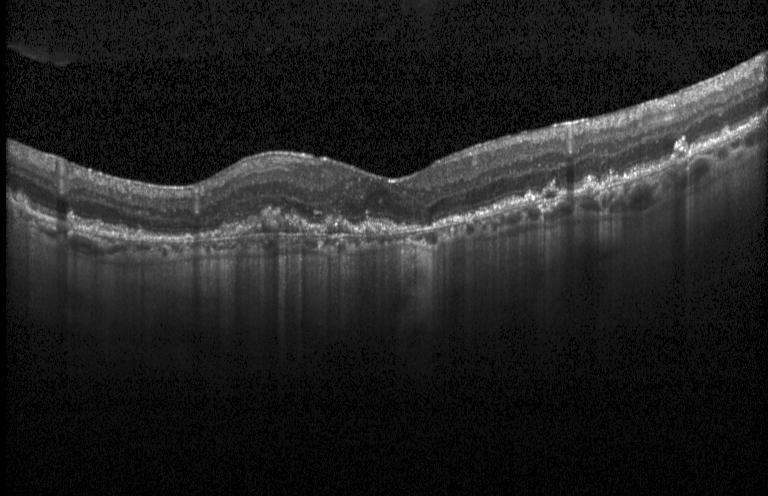

Optical coherence tomography B-scan.
Assessment: CNV.